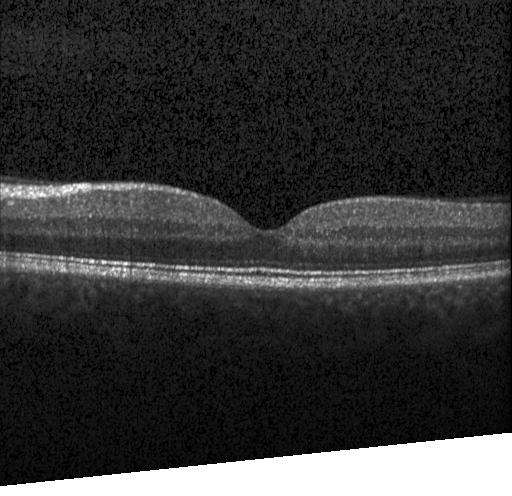
Macular OCT: no CNV, DME, or drusen.